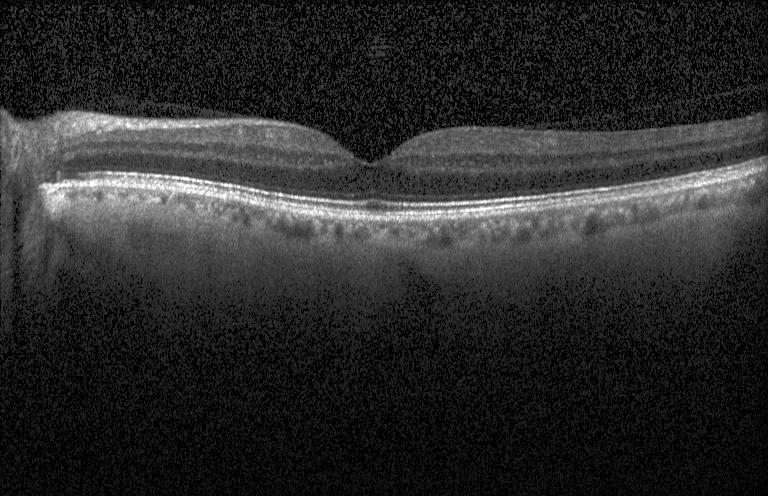

OCT finding: no CNV, DME, or drusen.